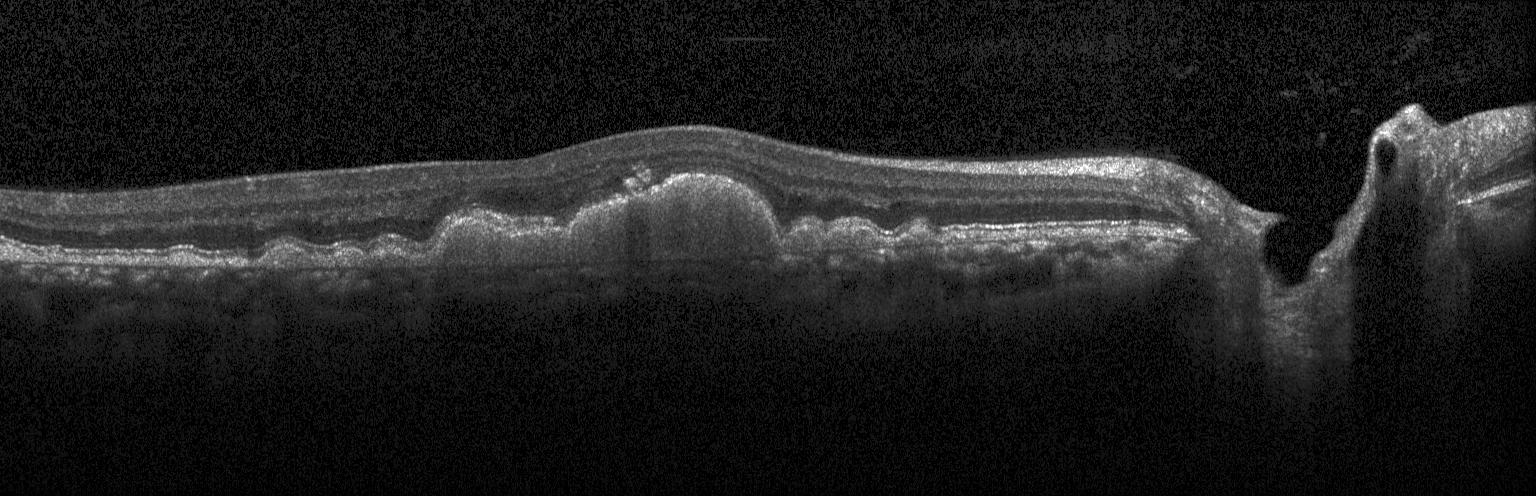 Impression: drusen.